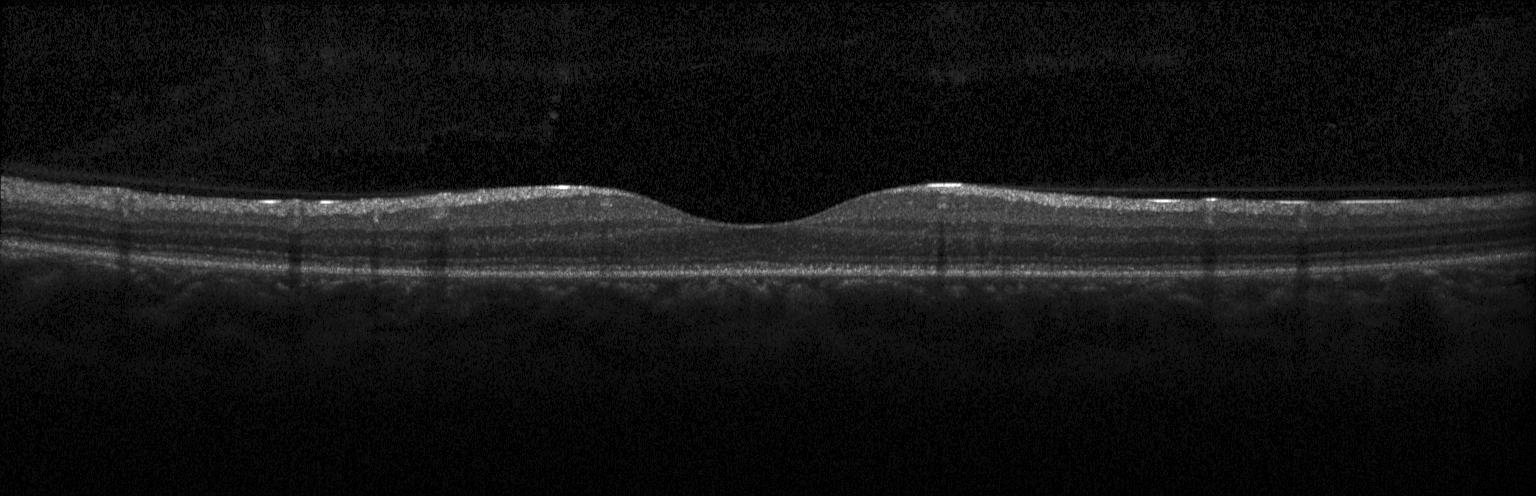

Retinal OCT B-scan, Heidelberg Spectralis OCT system, macular scan. Dx: no choroidal neovascularization, no diabetic macular edema, and no drusen.